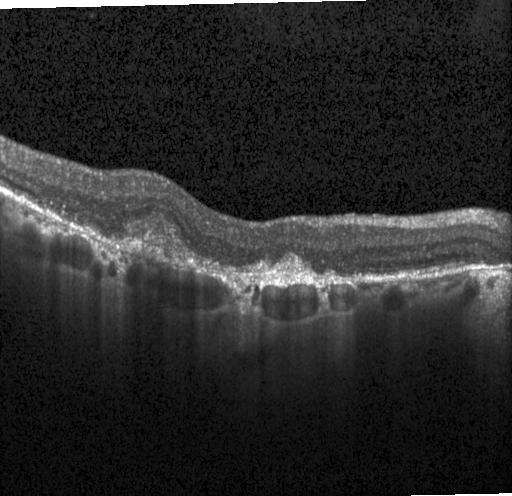

Impression: a choroidal neovascular membrane.